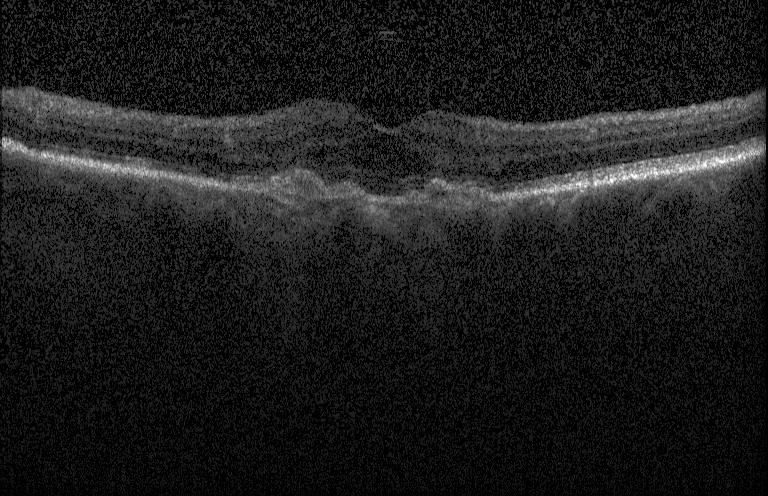

OCT line scan — Impression: choroidal neovascularization (CNV).